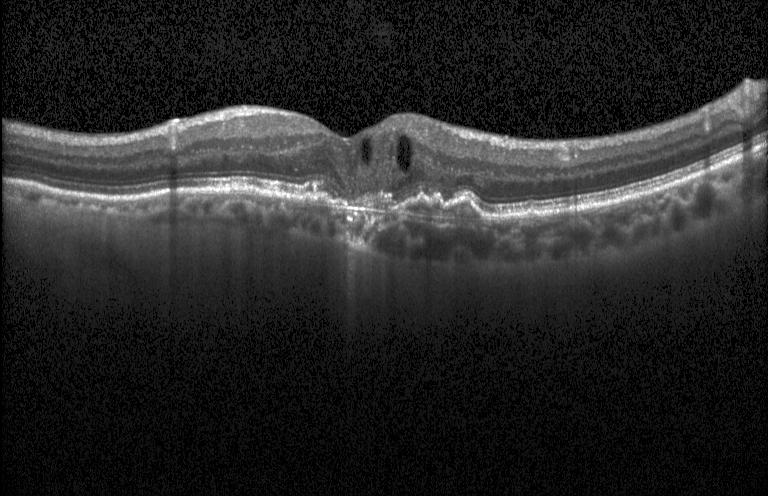

Optical coherence tomography B-scan, spectral-domain optical coherence tomography, instrument: Heidelberg Spectralis, centered on the fovea.
Impression: CNV.